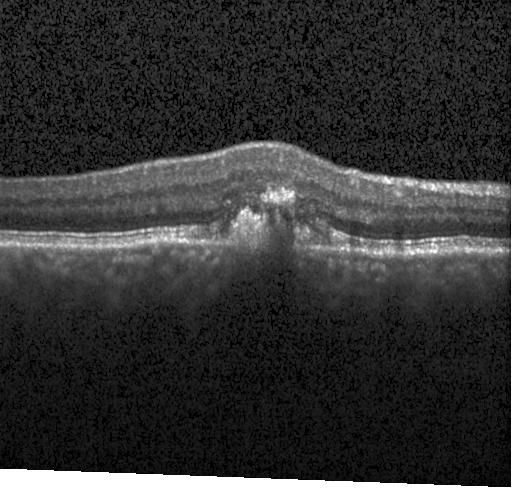 Diagnosis: CNV.